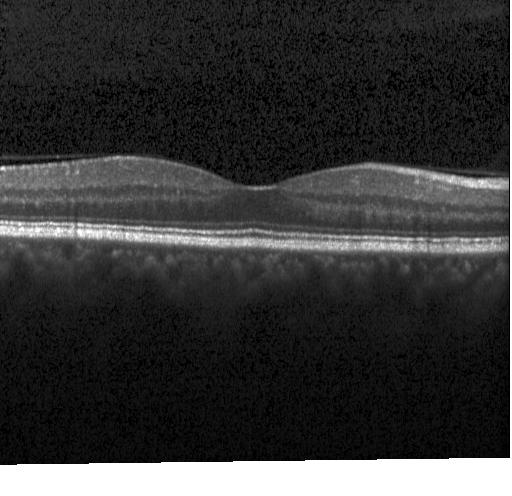

Optical coherence tomography scan — Impression: no choroidal neovascularization, diabetic macular edema, or drusen.